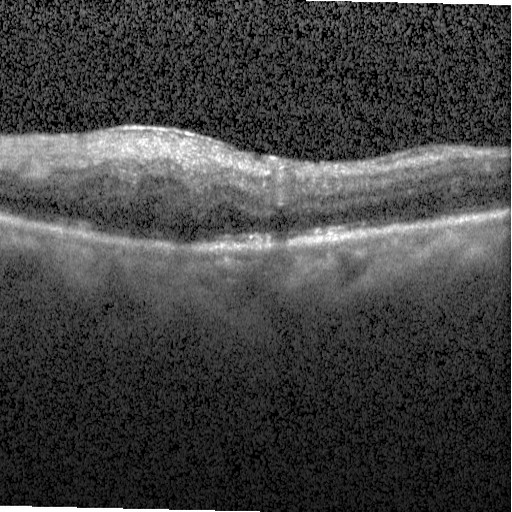 Retinal OCT cross-section. Dx: DME.